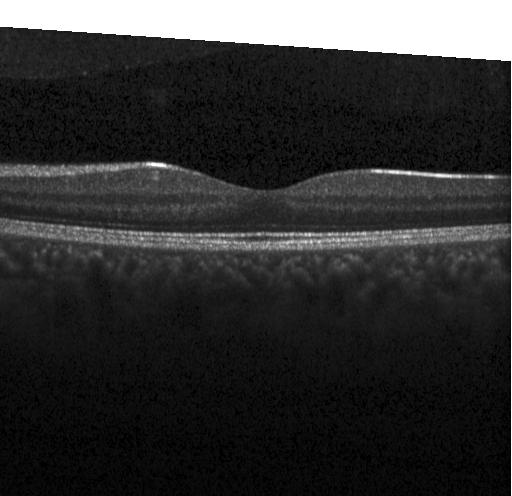

Optical coherence tomography scan, SD-OCT, Heidelberg Spectralis OCT system, macular scan — Finding: no CNV, DME, or drusen.